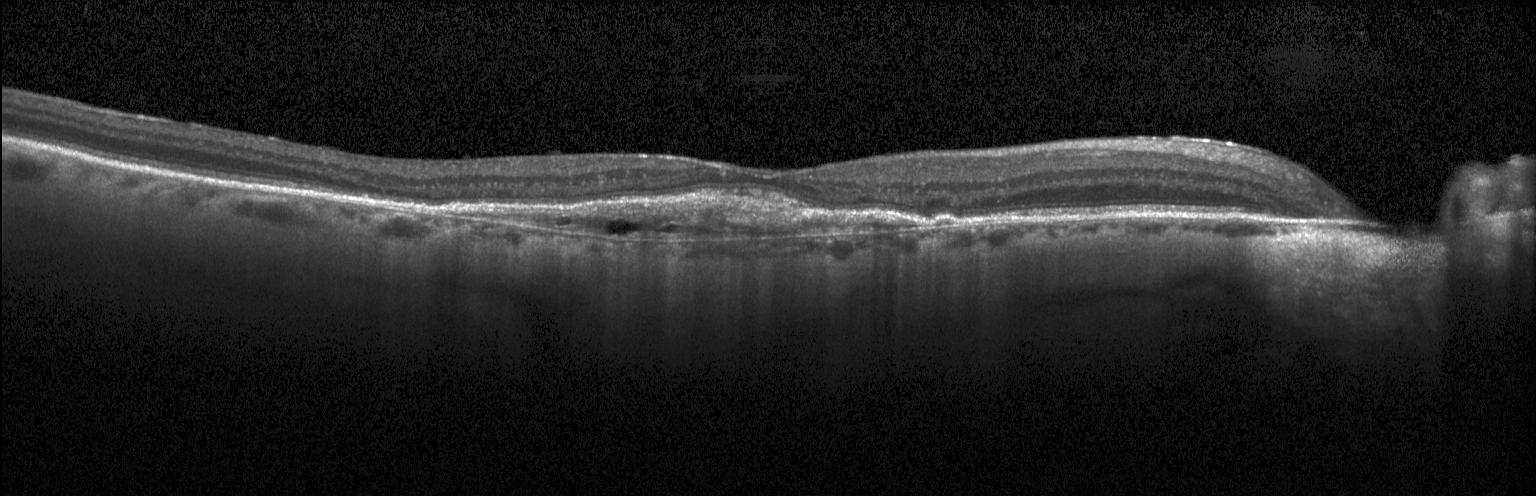
OCT line scan
Choroidal neovascularization.